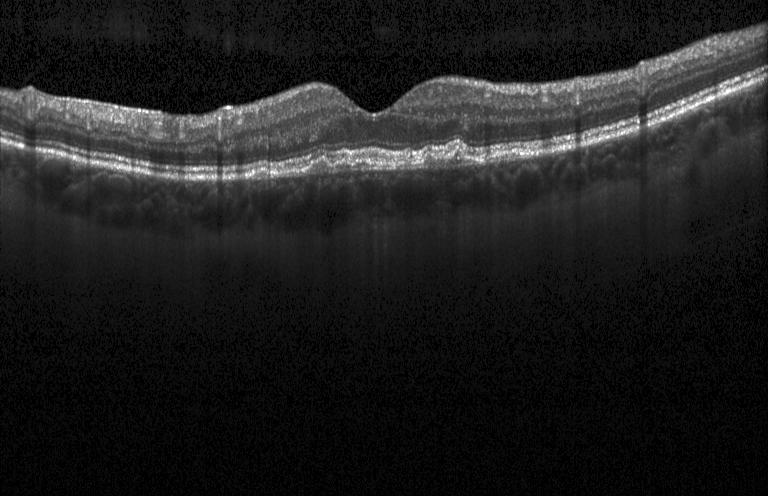
Dx: sub-RPE drusenoid deposits.